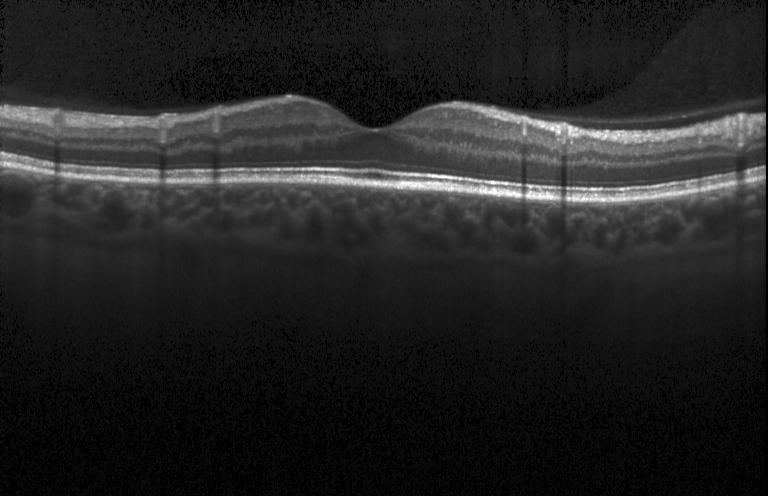 OCT B-scan. Macular OCT: neither choroidal neovascularization, diabetic macular edema, nor drusen.